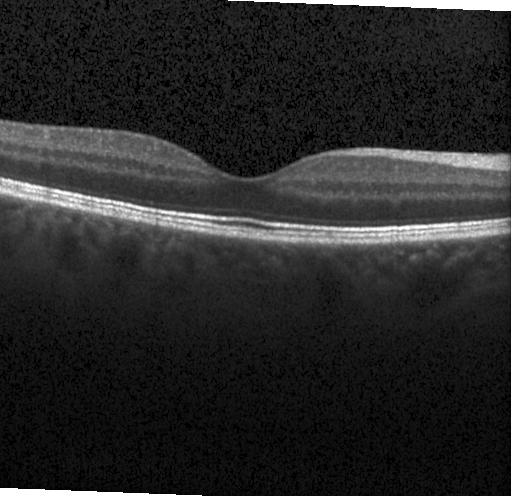 Heidelberg Spectralis OCT system. Retinal OCT B-scan.
OCT finding: no evidence of choroidal neovascularization, diabetic macular edema, or drusen.